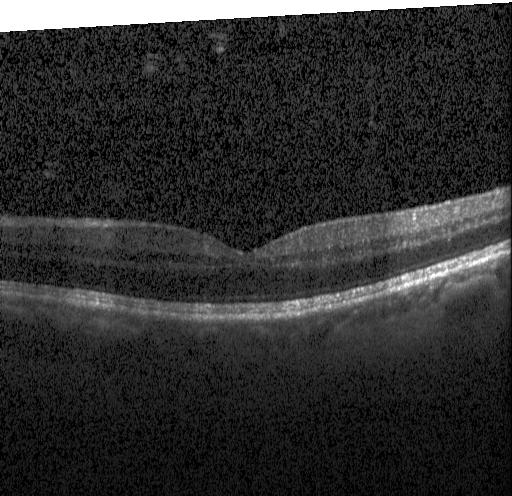

Macular scan · retinal OCT B-scan · spectral-domain optical coherence tomography · instrument: Heidelberg Spectralis
Diagnosis: no choroidal neovascularization, diabetic macular edema, or drusen.